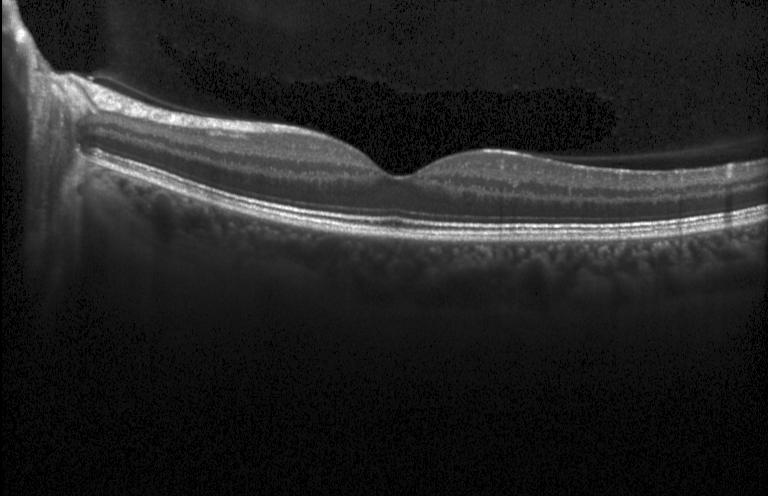 Acquired on a Heidelberg Spectralis, SD-OCT, horizontal scan through the fovea, optical coherence tomography B-scan
Dx: no evidence of choroidal neovascularization, diabetic macular edema, or drusen.